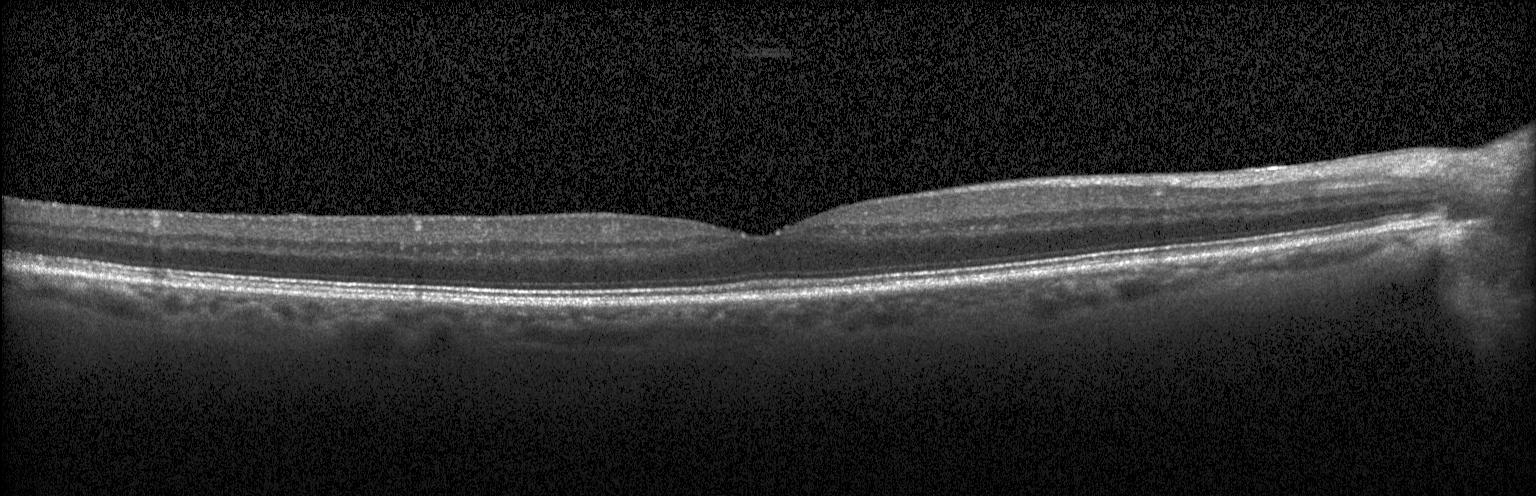
OCT finding: neither choroidal neovascularization, diabetic macular edema, nor drusen.